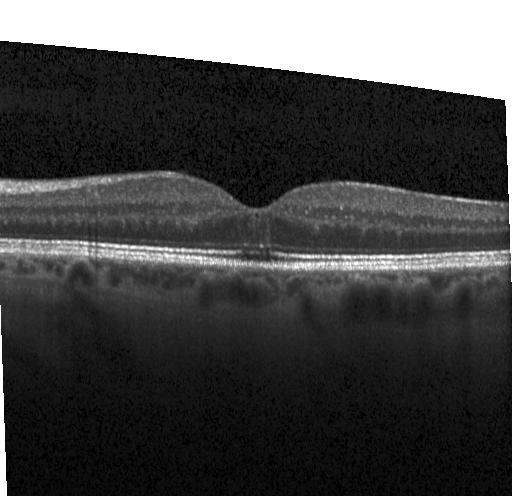 Impression: no choroidal neovascularization, no diabetic macular edema, and no drusen.